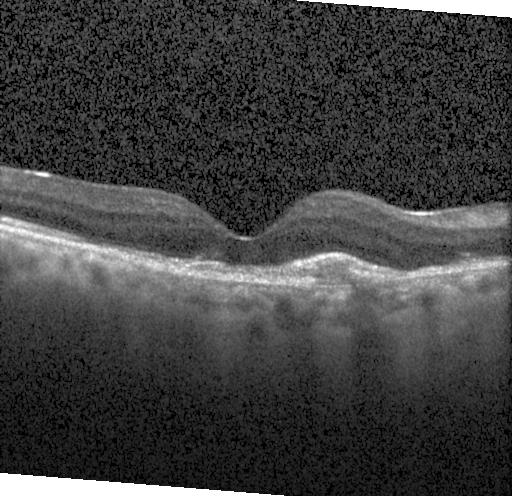
Finding: choroidal neovascularization (CNV).